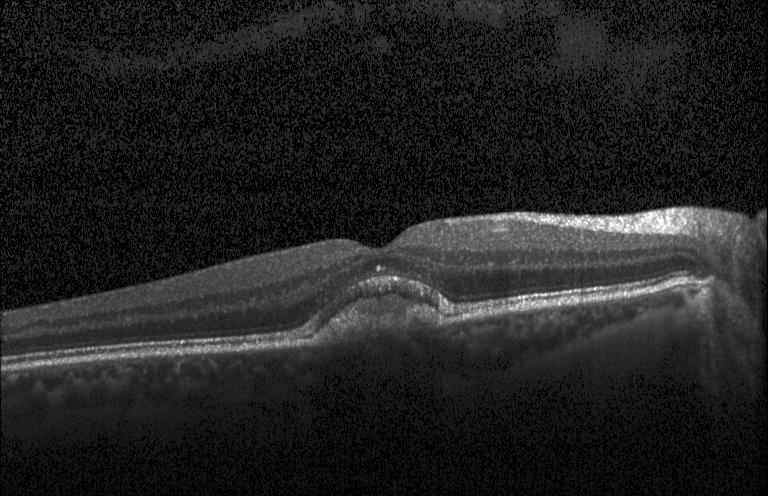 Optical coherence tomography scan — Choroidal neovascularization (CNV).